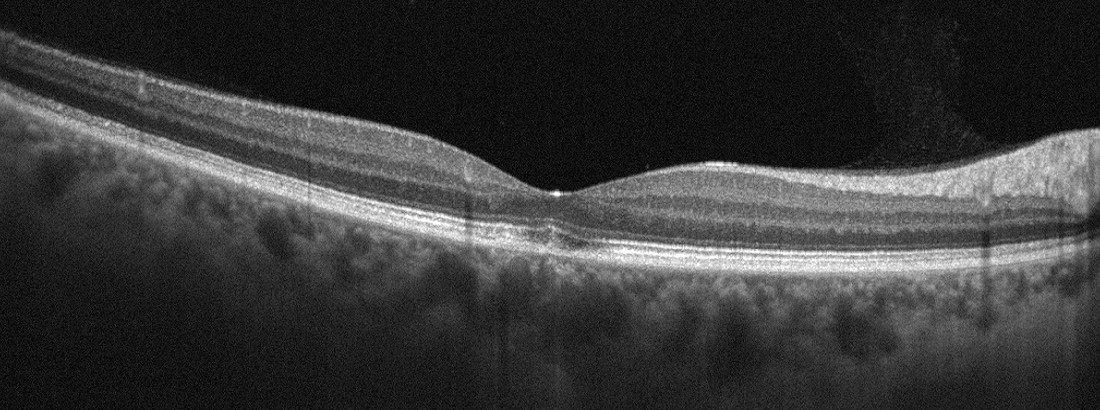 Instrument: Optovue Avanti RTVue XR · retinal OCT cross-section · macular scan. Finding: age-related macular degeneration.